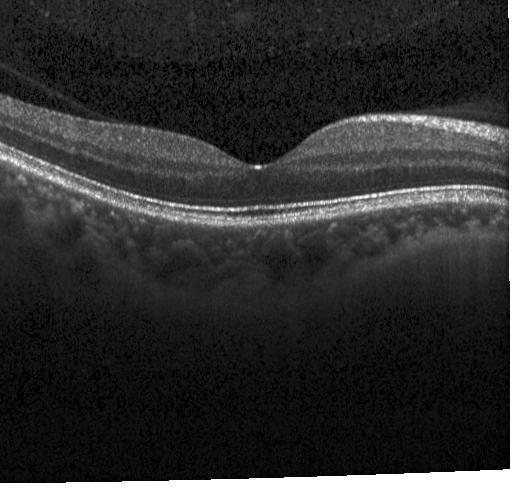 Optical coherence tomography scan.
The scan shows no CNV, DME, or drusen.